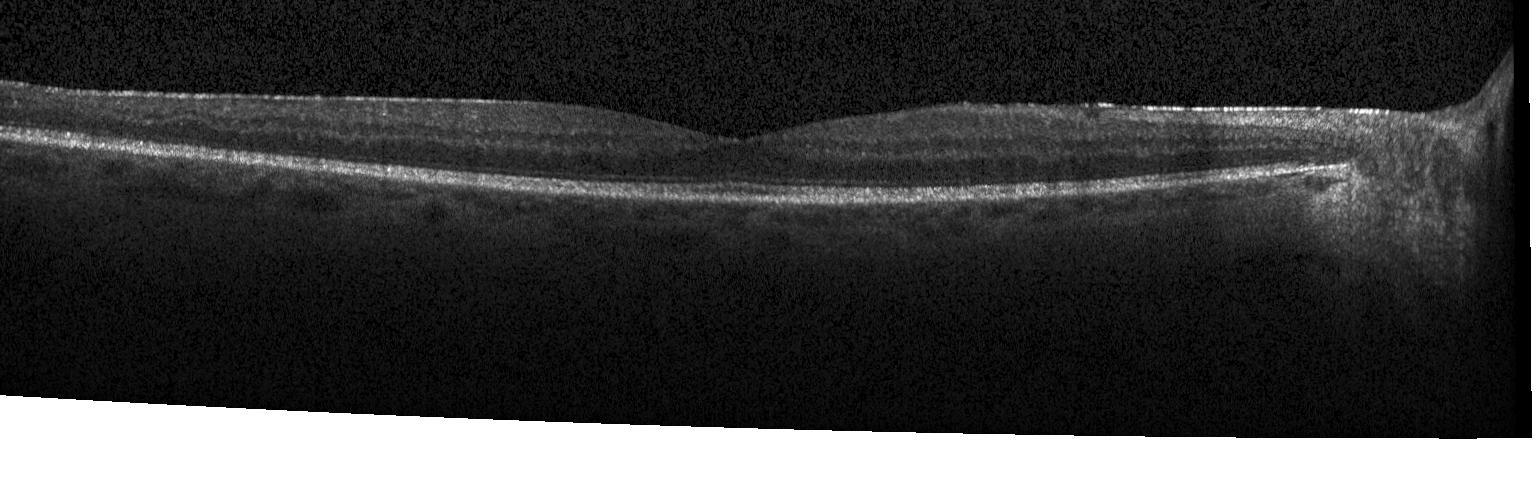
Acquired on a Heidelberg Spectralis; optical coherence tomography scan
This B-scan demonstrates neither choroidal neovascularization, diabetic macular edema, nor drusen.